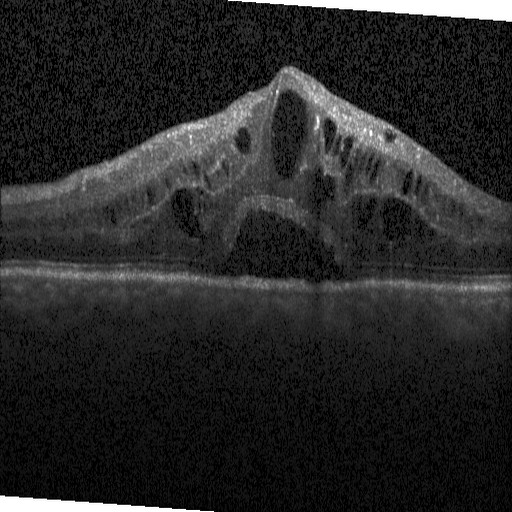
Retinal OCT B-scan.
Dx: DME.